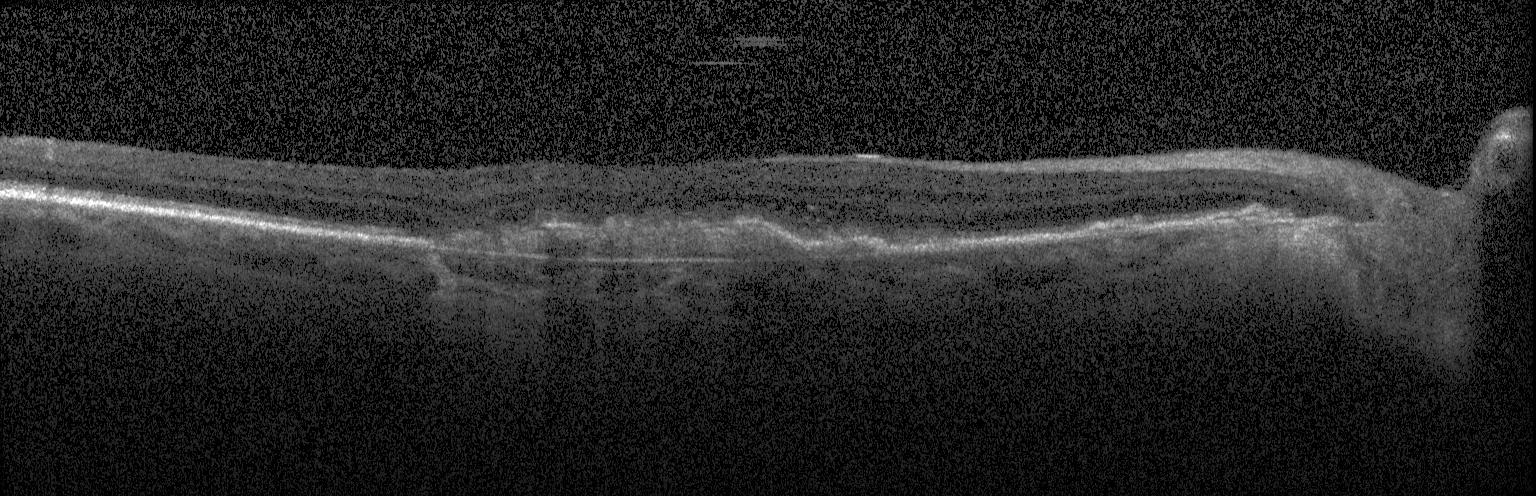
This B-scan demonstrates choroidal neovascularization.